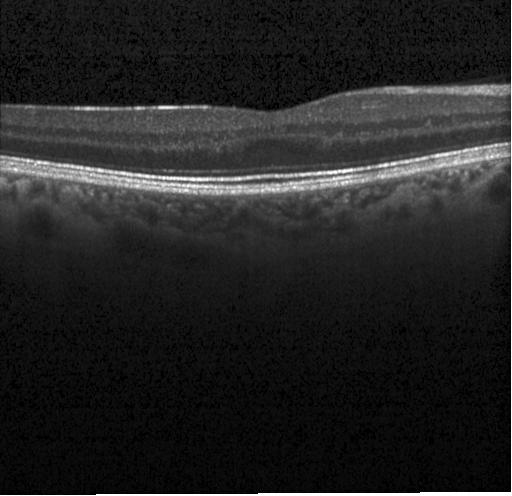
OCT scan showing no choroidal neovascularization, diabetic macular edema, or drusen.